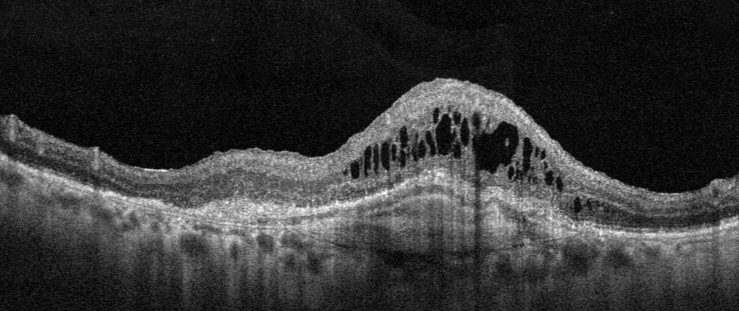
OCT B-scan; acquired on an Optovue Avanti RTVue XR. Dx: AMD.